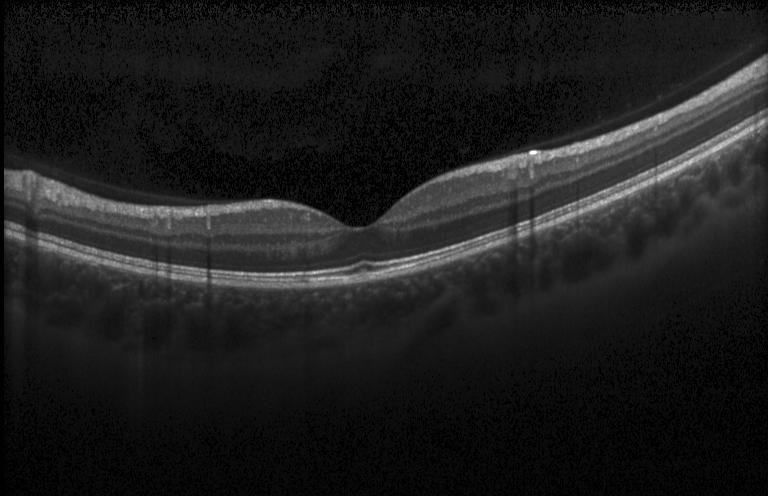
Fovea-centered, OCT B-scan, spectral-domain optical coherence tomography — This B-scan demonstrates neither choroidal neovascularization, diabetic macular edema, nor drusen.